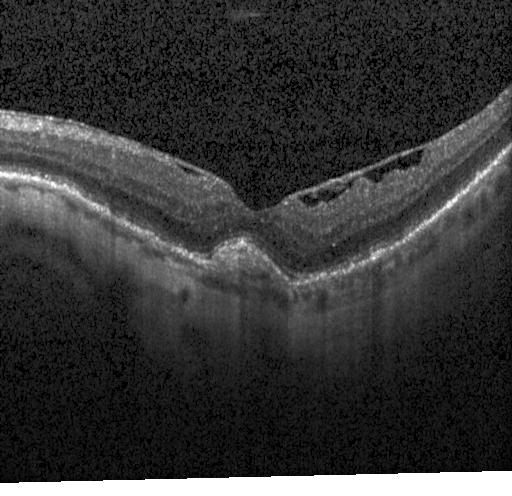

Spectral-domain optical coherence tomography · OCT B-scan — Macular OCT: a choroidal neovascular membrane.